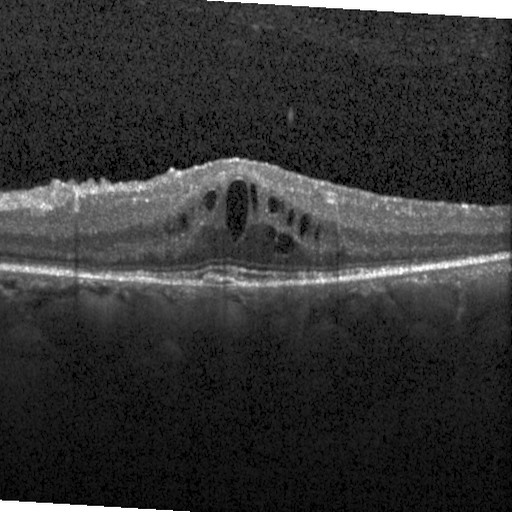
Optical coherence tomography B-scan. Diagnosis: diabetic macular edema (DME).